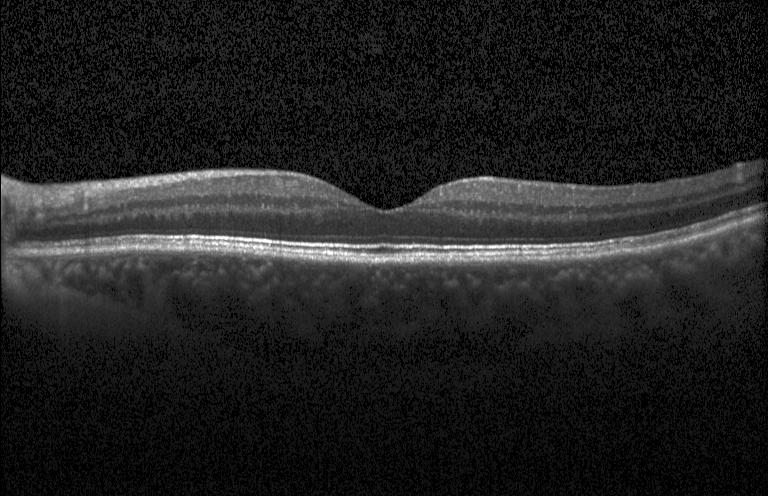
OCT line scan.
Finding: no choroidal neovascularization, diabetic macular edema, or drusen.